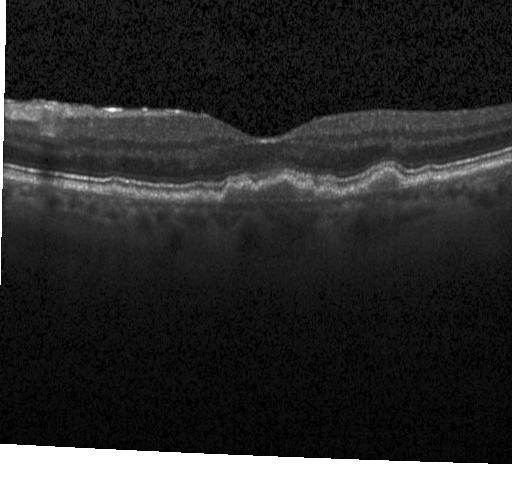

Macular OCT: multiple drusen.